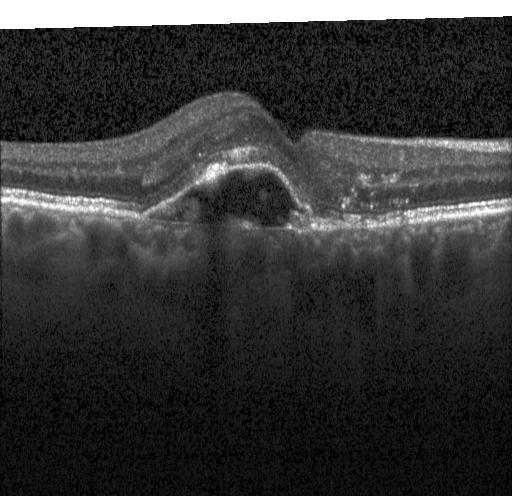
Finding: a choroidal neovascular membrane.